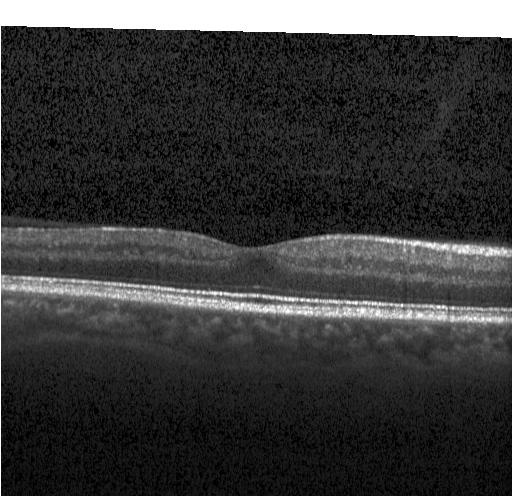
Optical coherence tomography scan, spectral-domain optical coherence tomography, Heidelberg Spectralis OCT system — Diagnosis: neither CNV, DME, nor drusen.